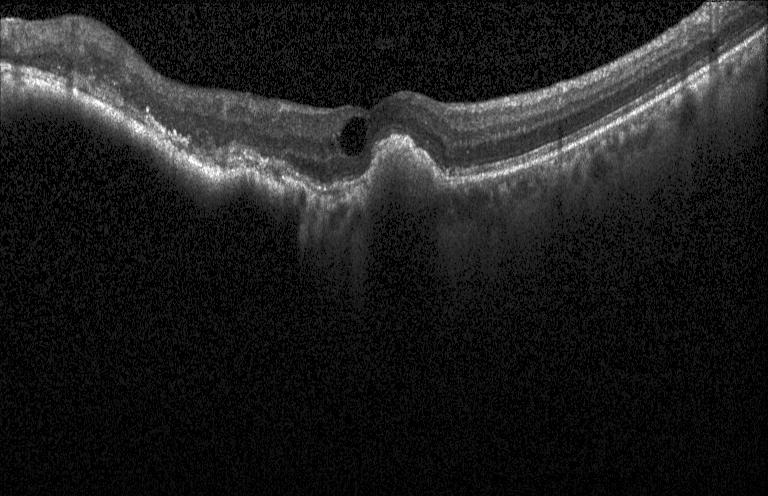 OCT finding: CNV.